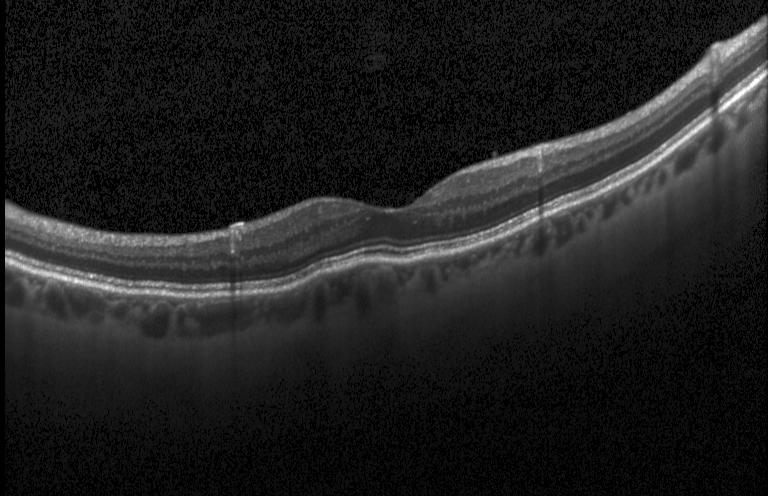

Optical coherence tomography scan, spectral-domain optical coherence tomography, centered on the fovea, acquired on a Heidelberg Spectralis. Impression: no evidence of choroidal neovascularization, diabetic macular edema, or drusen.